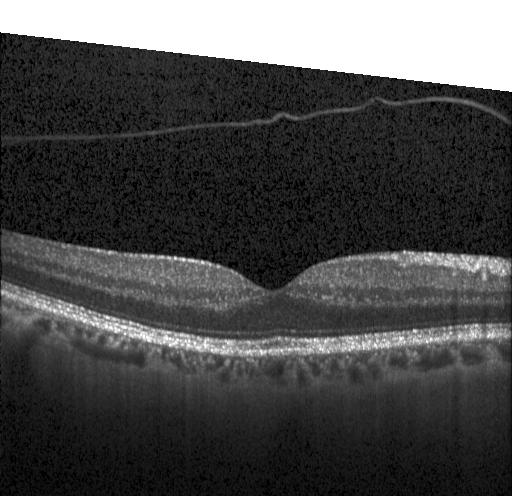 No choroidal neovascularization, diabetic macular edema, or drusen.